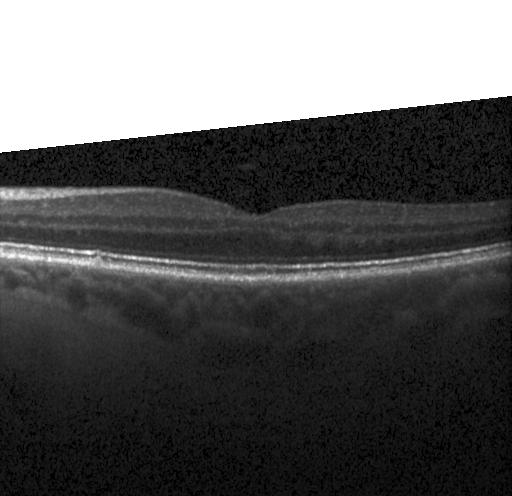
Assessment: sub-RPE drusenoid deposits.